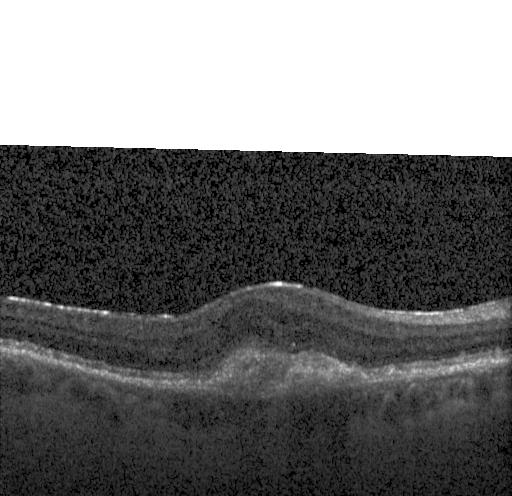

OCT B-scan — Impression: choroidal neovascularization (CNV).